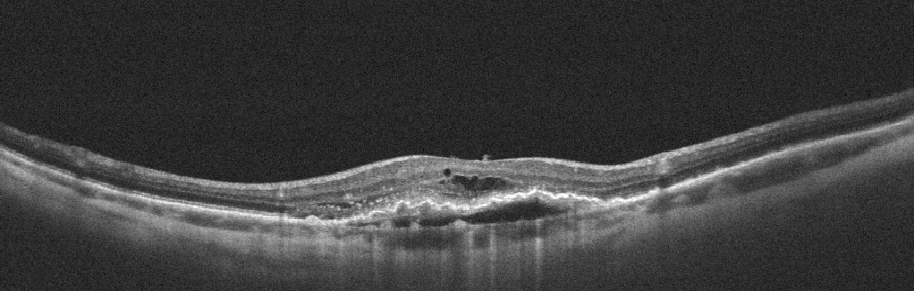
Instrument: Optovue Avanti RTVue XR, left eye, retinal OCT cross-section — OCT finding: AMD.